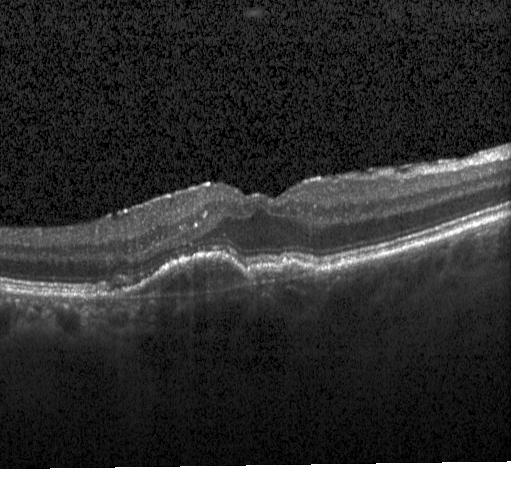
The scan shows a choroidal neovascular membrane.